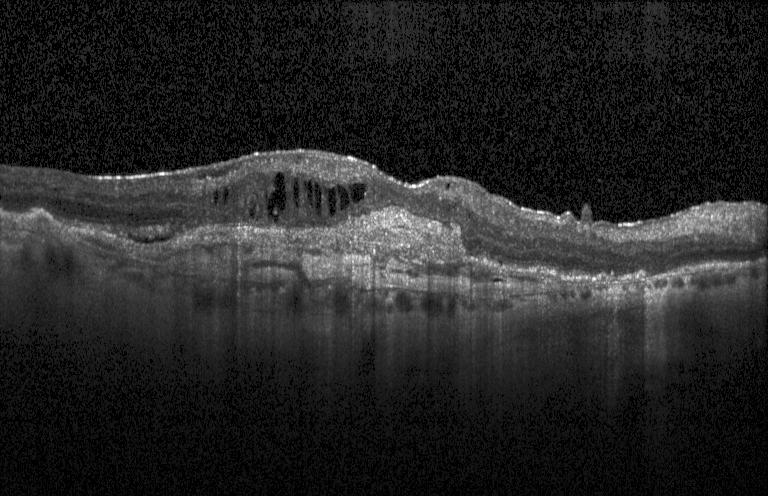

Retinal OCT B-scan · spectral-domain OCT — Impression: choroidal neovascularization (CNV).